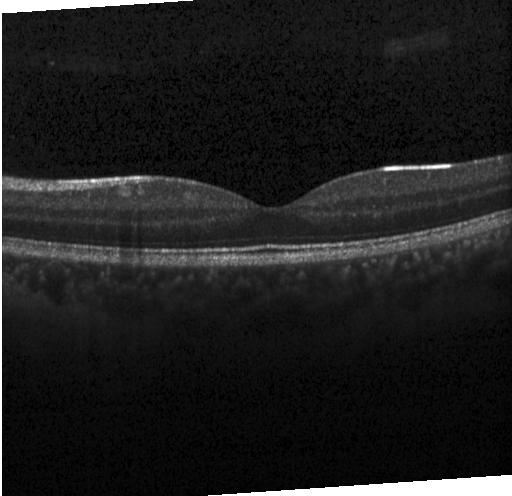 Retinal OCT B-scan — Finding: no evidence of CNV, DME, or drusen.